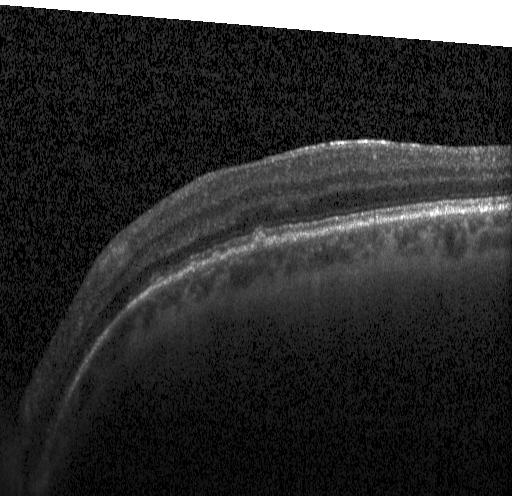

Macular OCT: sub-RPE drusenoid deposits.